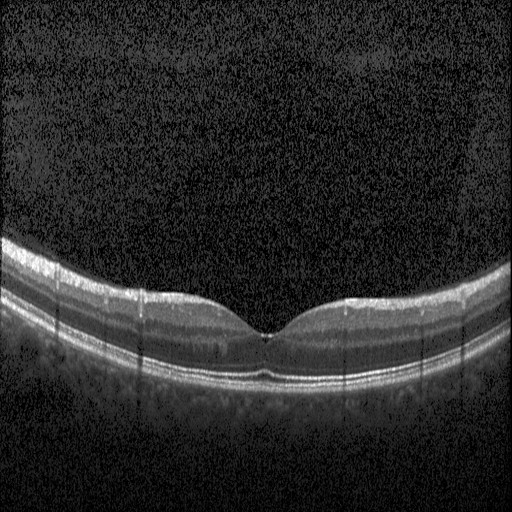

Retinal OCT B-scan, spectral-domain optical coherence tomography, horizontal scan through the fovea — Diabetic macular edema.